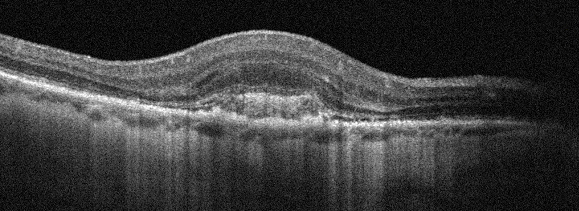
Oculus dexter · optical coherence tomography B-scan. Diagnosis: AMD.